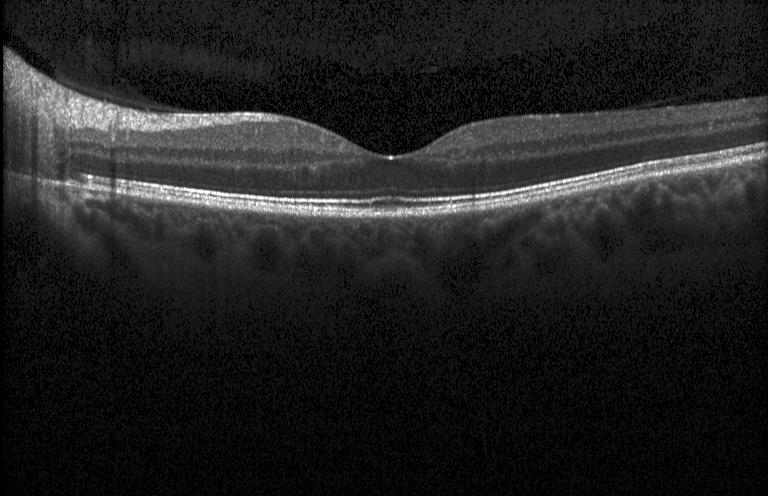 Spectral-domain OCT · optical coherence tomography scan · acquired on a Heidelberg Spectralis · through the macula — Macular OCT: no choroidal neovascularization, diabetic macular edema, or drusen.